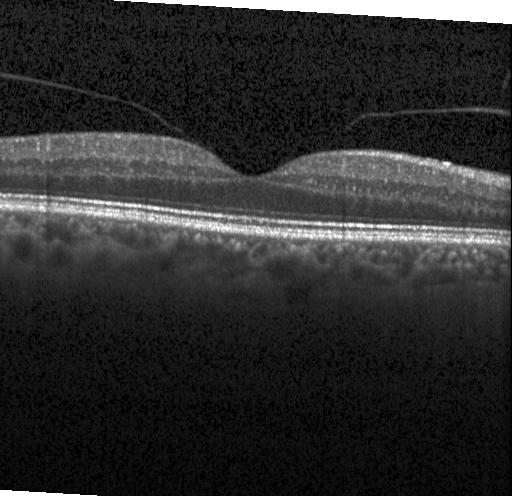

SD-OCT. Through the macula. Heidelberg Spectralis OCT system. Retinal OCT cross-section
The scan shows no CNV, no DME, and no drusen.